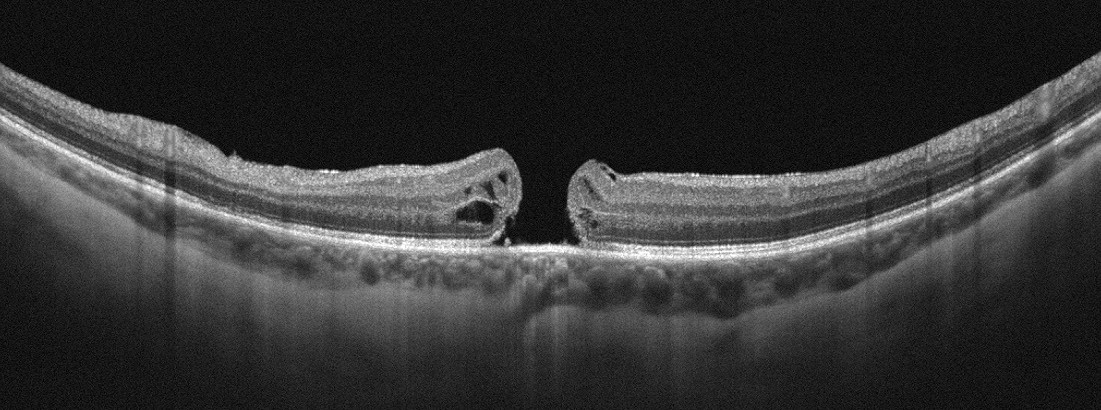

Optical coherence tomography B-scan. The scan shows VID.